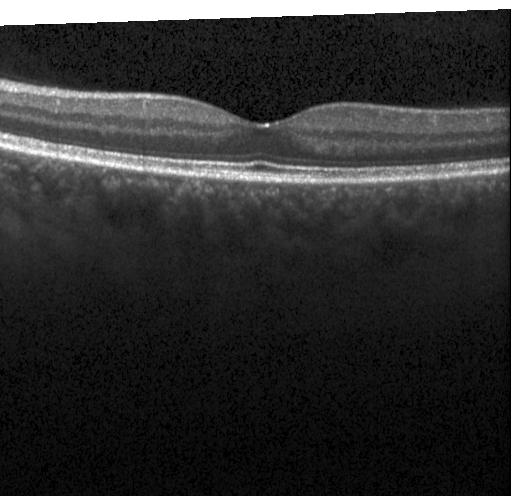 OCT B-scan. SD-OCT. Instrument: Heidelberg Spectralis. Macular scan. Finding: neither choroidal neovascularization, diabetic macular edema, nor drusen.